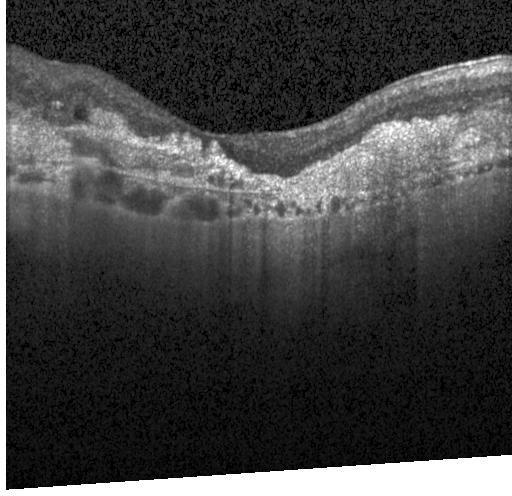
Optical coherence tomography scan. Spectral-domain optical coherence tomography — OCT finding: CNV.